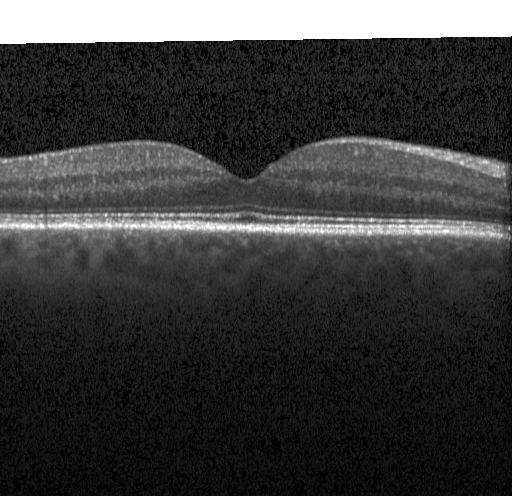 OCT scan showing no evidence of choroidal neovascularization, diabetic macular edema, or drusen.